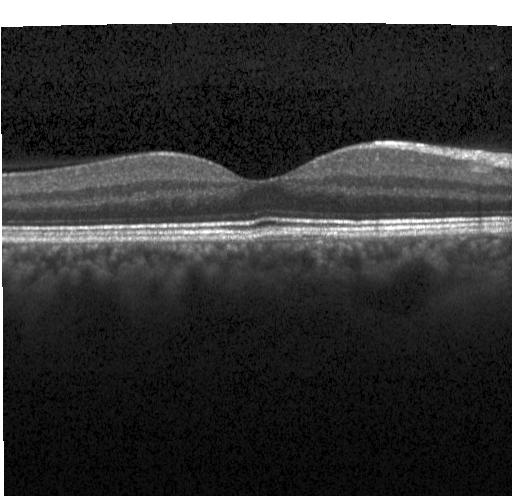
Retinal OCT B-scan, horizontal scan through the fovea, spectral-domain OCT
This B-scan demonstrates neither choroidal neovascularization, diabetic macular edema, nor drusen.